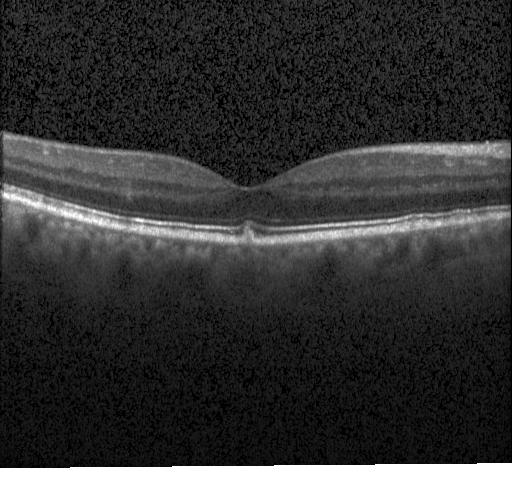

Impression: drusen.